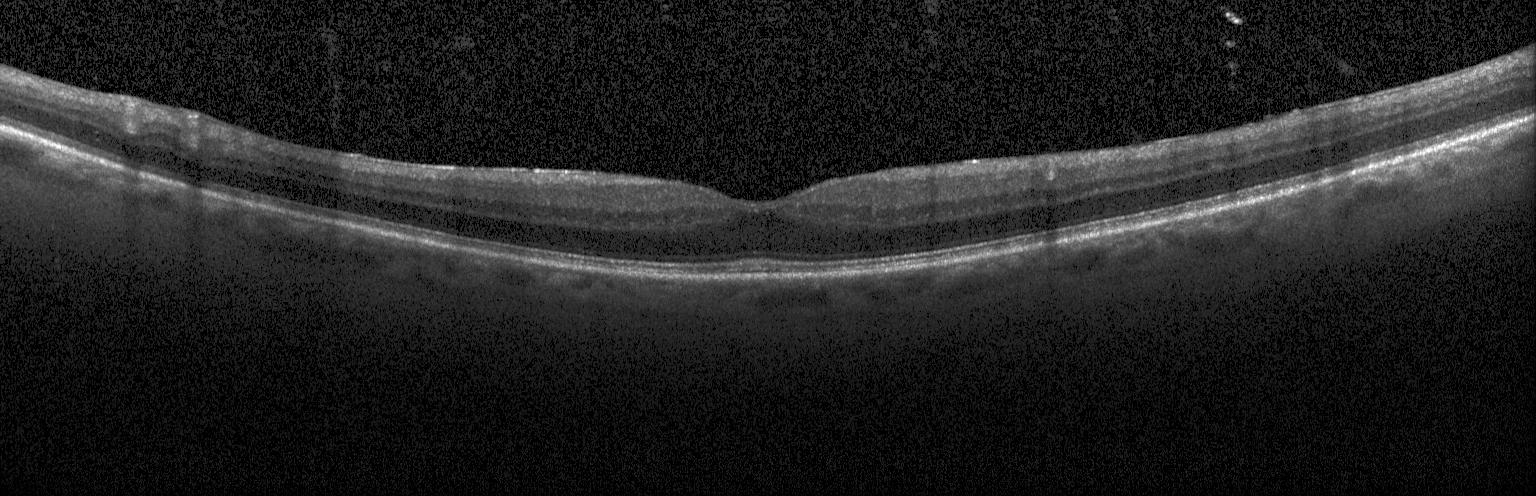
Spectral-domain optical coherence tomography · OCT B-scan — Diagnosis: no evidence of choroidal neovascularization, diabetic macular edema, or drusen.